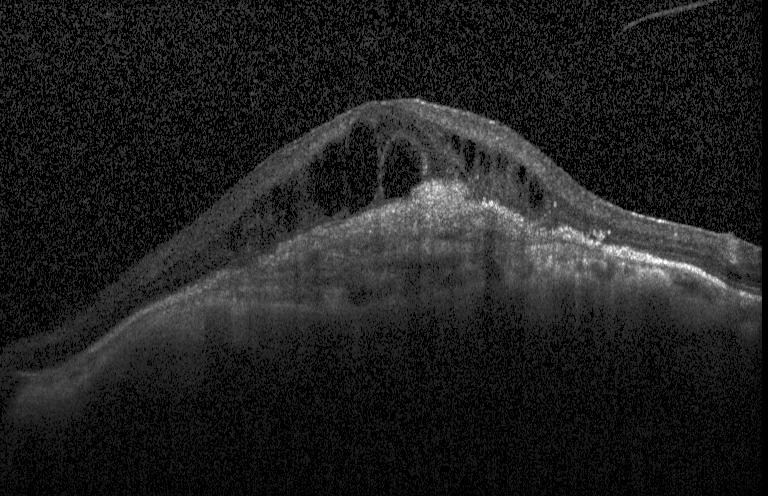 Optical coherence tomography B-scan. The scan shows choroidal neovascularization.